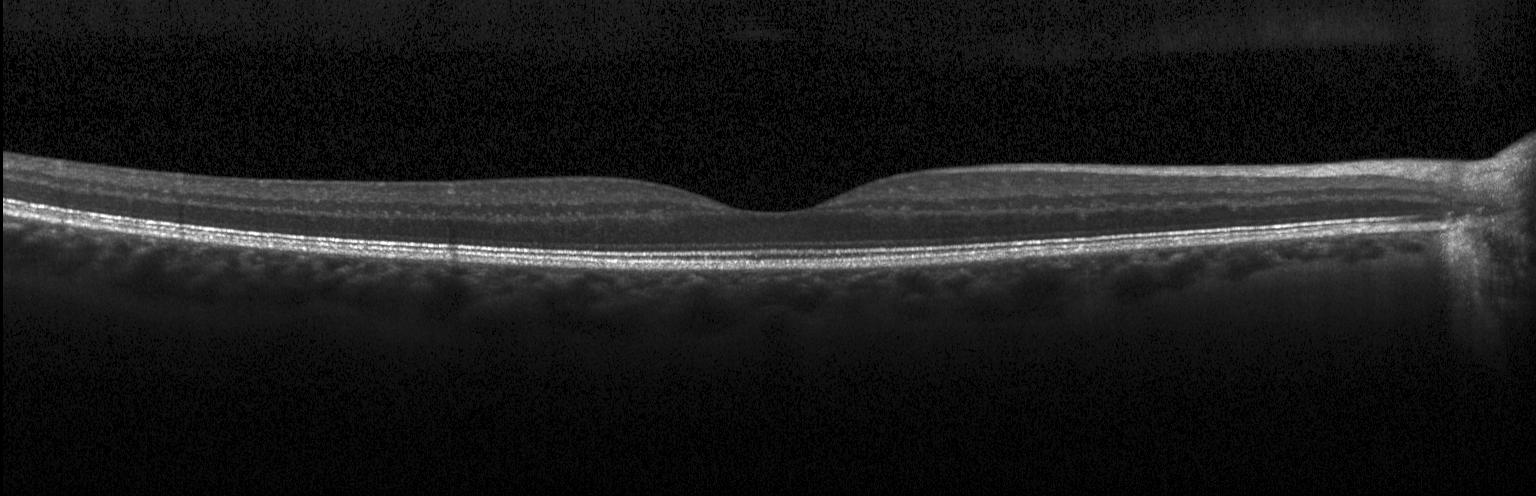 Optical coherence tomography B-scan — Finding: neither choroidal neovascularization, diabetic macular edema, nor drusen.